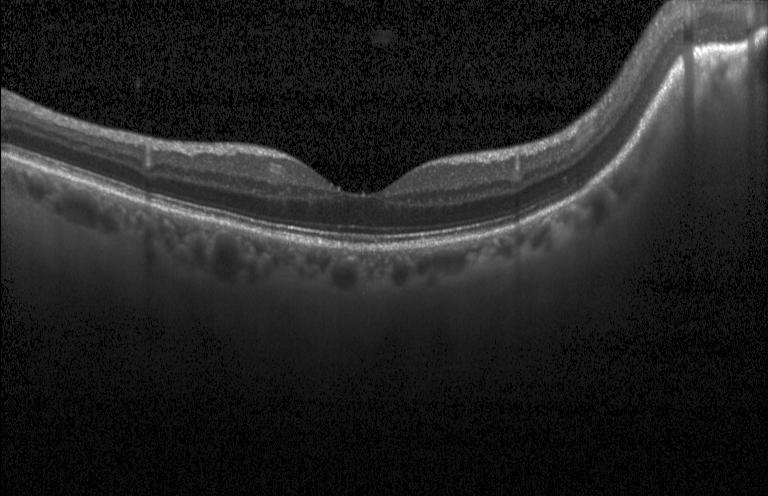
Heidelberg Spectralis OCT system · SD-OCT · optical coherence tomography scan · horizontal scan through the fovea.
Diagnosis: neither CNV, DME, nor drusen.